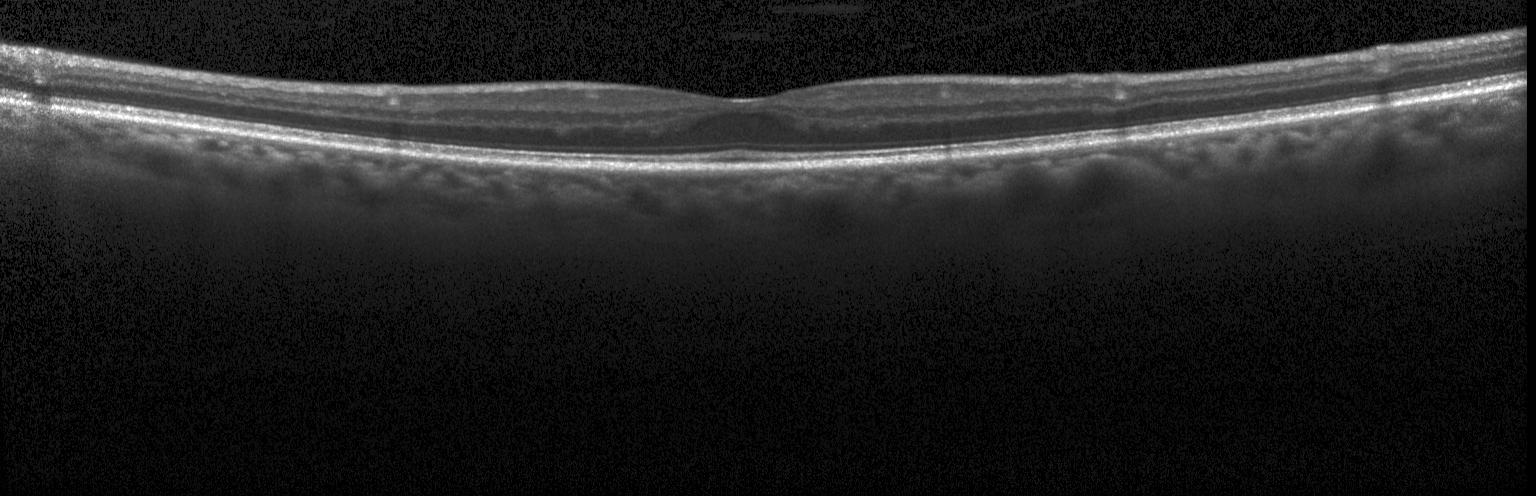 Diagnosis: no choroidal neovascularization, diabetic macular edema, or drusen.